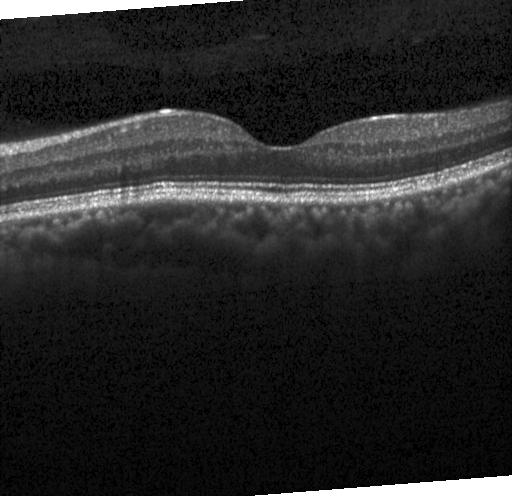

Heidelberg Spectralis, centered on the fovea, SD-OCT, OCT B-scan. Finding: no evidence of choroidal neovascularization, diabetic macular edema, or drusen.